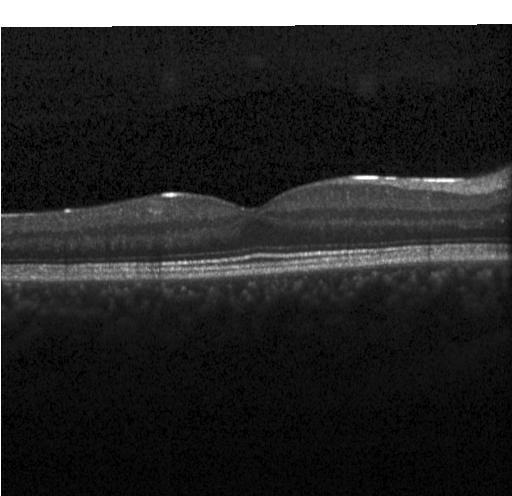 Retinal OCT B-scan. Heidelberg Spectralis OCT system
Macular OCT: neither CNV, DME, nor drusen.